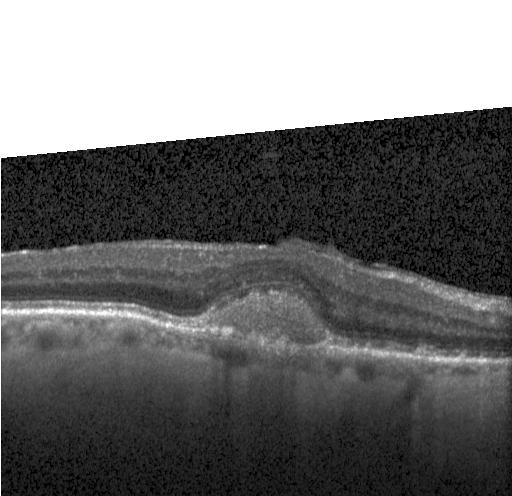 Optical coherence tomography B-scan; spectral-domain optical coherence tomography; acquired on a Heidelberg Spectralis; through the macula
Diagnosis: a choroidal neovascular membrane.